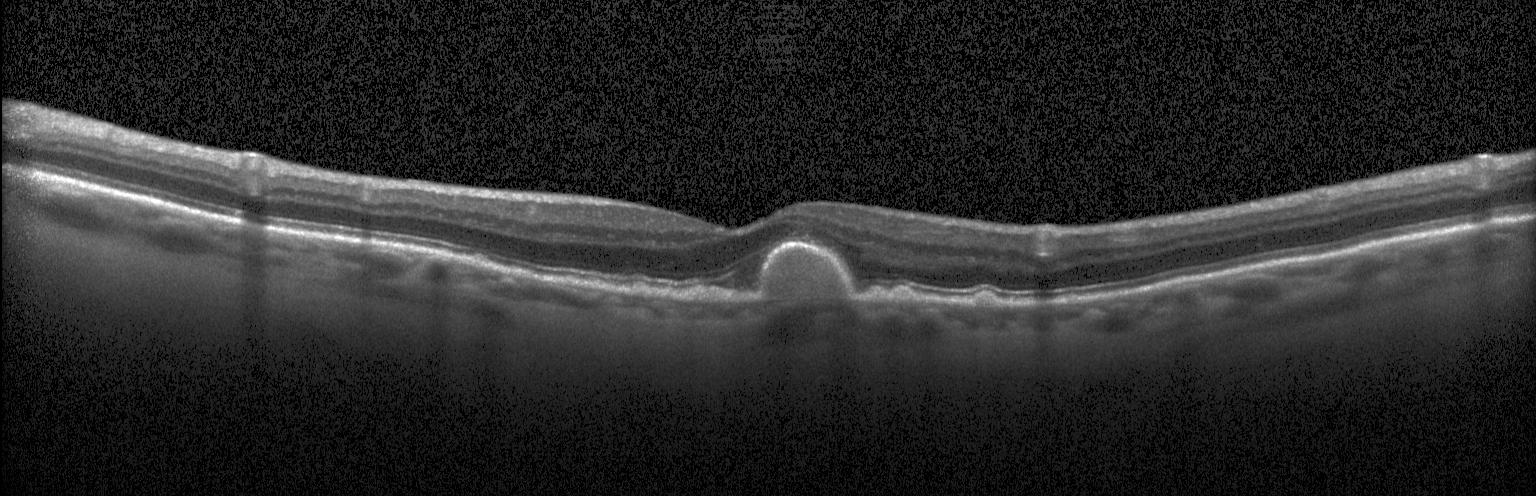
Optical coherence tomography scan
Impression: drusen.